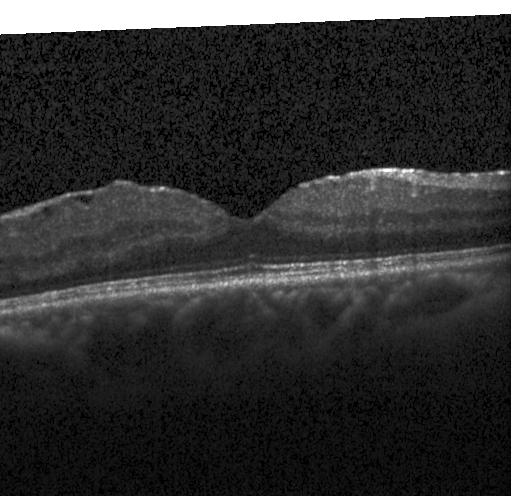

Heidelberg Spectralis OCT system; horizontal scan through the fovea; OCT B-scan.
Finding: neither choroidal neovascularization, diabetic macular edema, nor drusen.